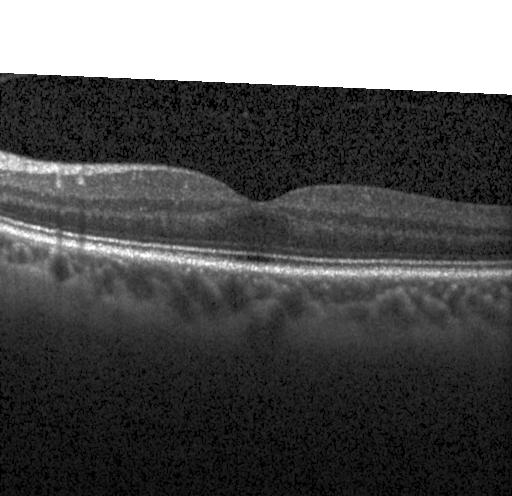

Macular scan · Heidelberg Spectralis OCT system · OCT B-scan — Assessment: neither choroidal neovascularization, diabetic macular edema, nor drusen.